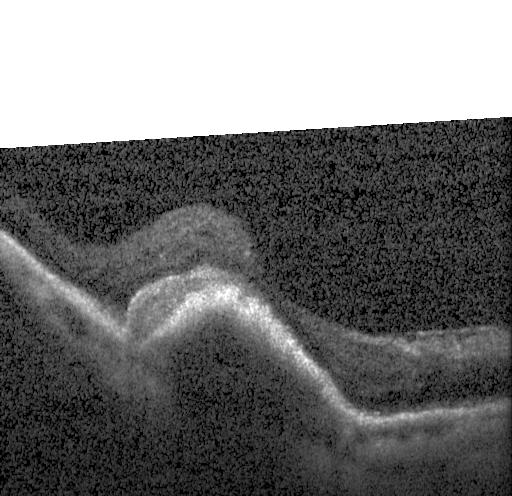
Heidelberg Spectralis, spectral-domain optical coherence tomography, OCT B-scan — Dx: a choroidal neovascular membrane.